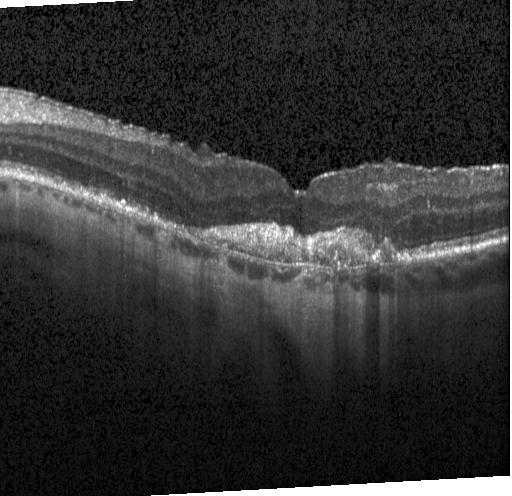
Retinal OCT cross-section. Finding: choroidal neovascularization.